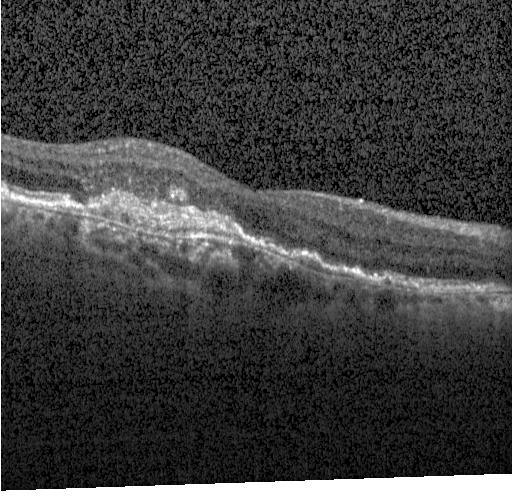

Spectral-domain OCT B-scan: a choroidal neovascular membrane.